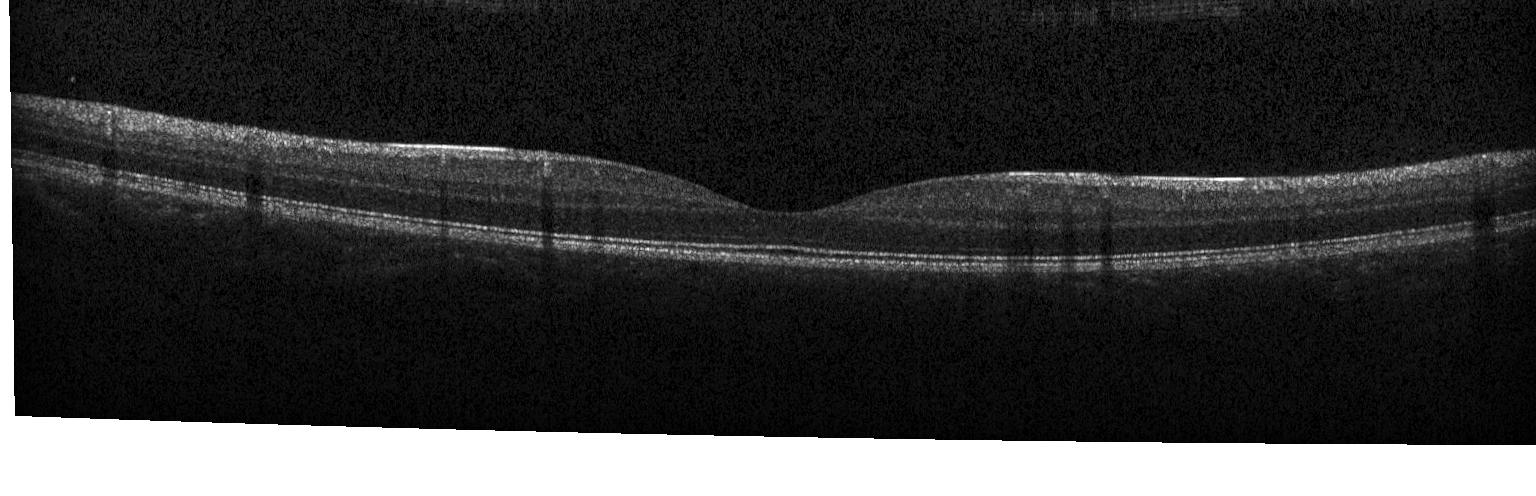
Spectral-domain optical coherence tomography. Retinal OCT cross-section. Centered on the fovea.
Assessment: no evidence of choroidal neovascularization, diabetic macular edema, or drusen.